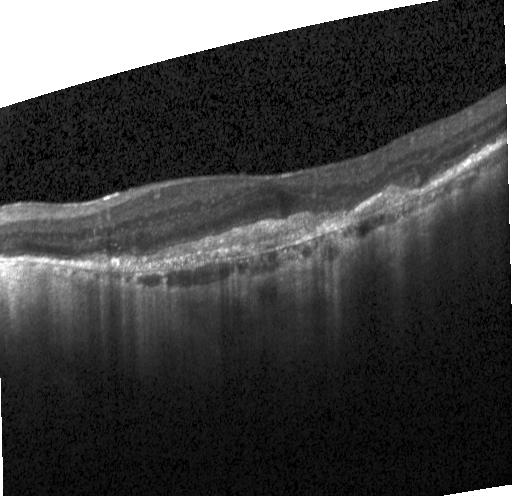
OCT scan showing a choroidal neovascular membrane.